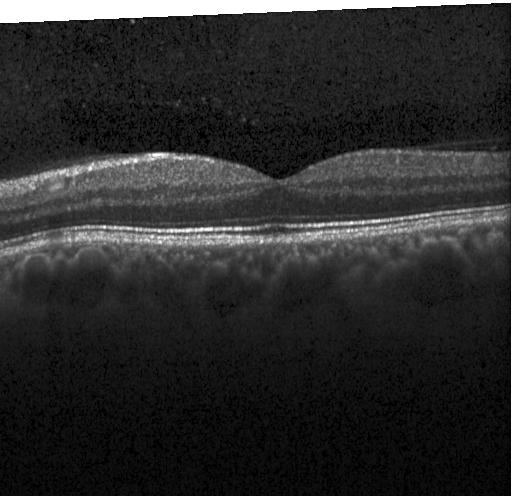

Optical coherence tomography B-scan.
Dx: no choroidal neovascularization, diabetic macular edema, or drusen.